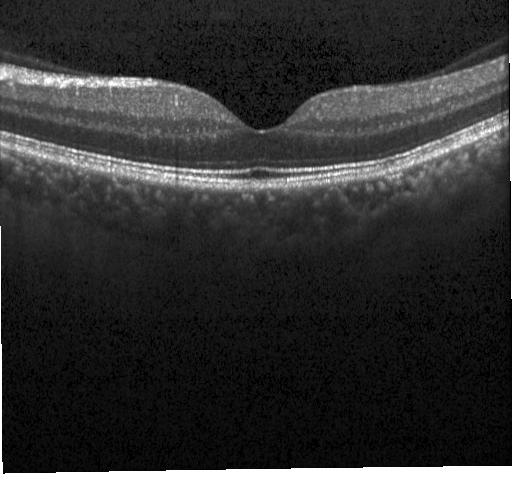 Optical coherence tomography B-scan, horizontal scan through the fovea — Macular OCT: no choroidal neovascularization, diabetic macular edema, or drusen.